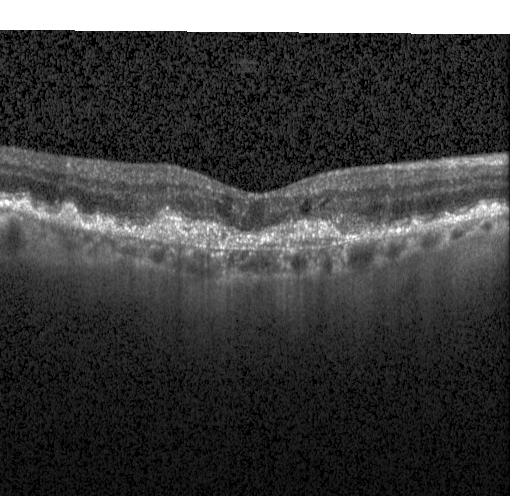

Impression: CNV.